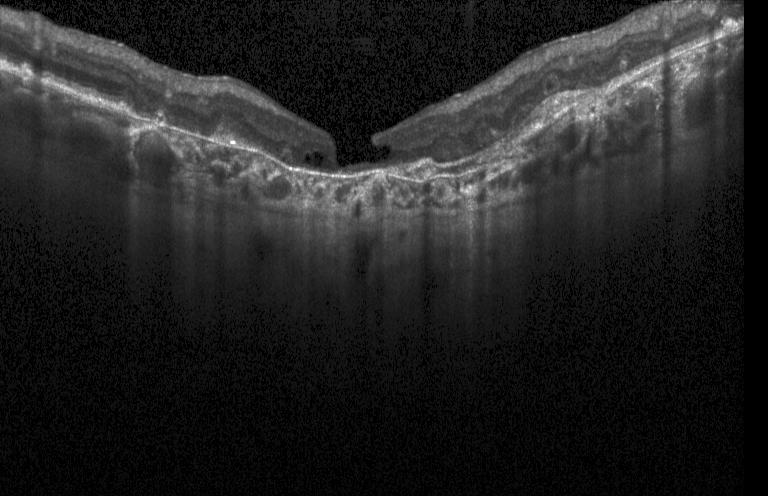
Optical coherence tomography B-scan; fovea-centered
Dx: choroidal neovascularization (CNV).